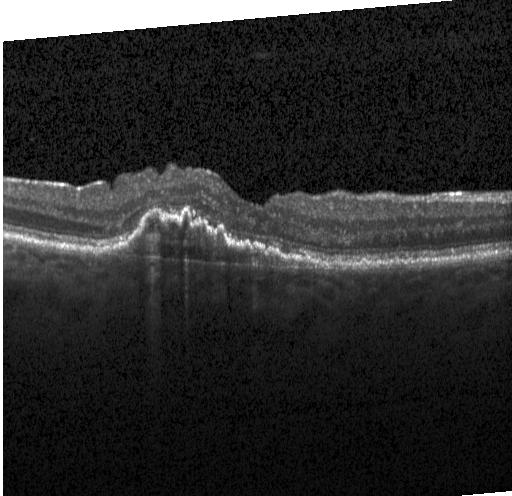
Optical coherence tomography B-scan · spectral-domain OCT. The scan shows CNV.